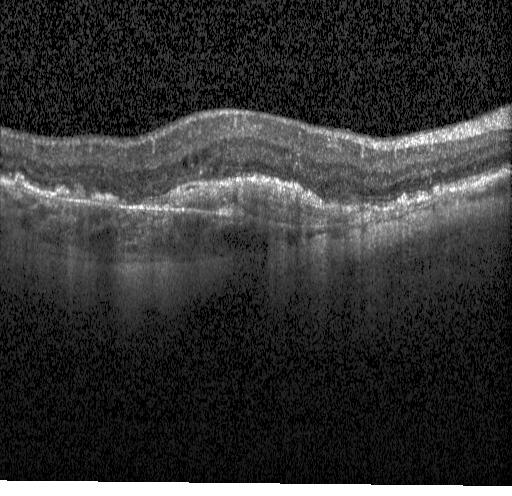 The scan shows choroidal neovascularization.